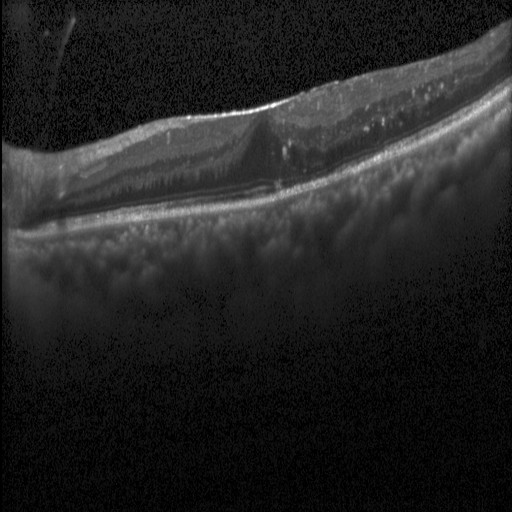 Optical coherence tomography scan · macular scan · spectral-domain OCT.
DME.